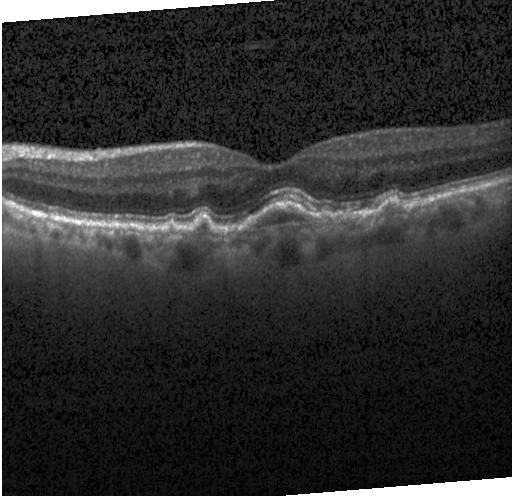

Spectral-domain optical coherence tomography · Heidelberg Spectralis · optical coherence tomography B-scan. Finding: a choroidal neovascular membrane.